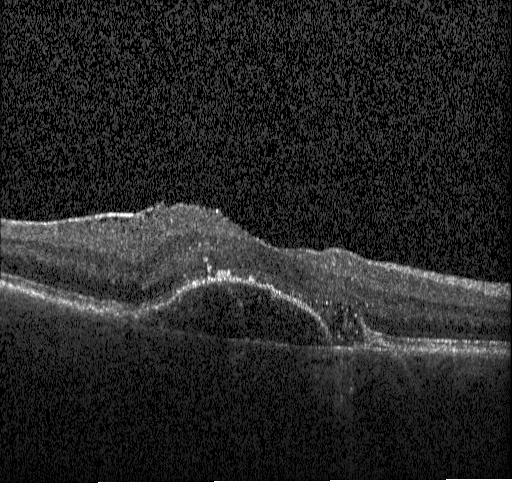
The scan shows choroidal neovascularization (CNV).